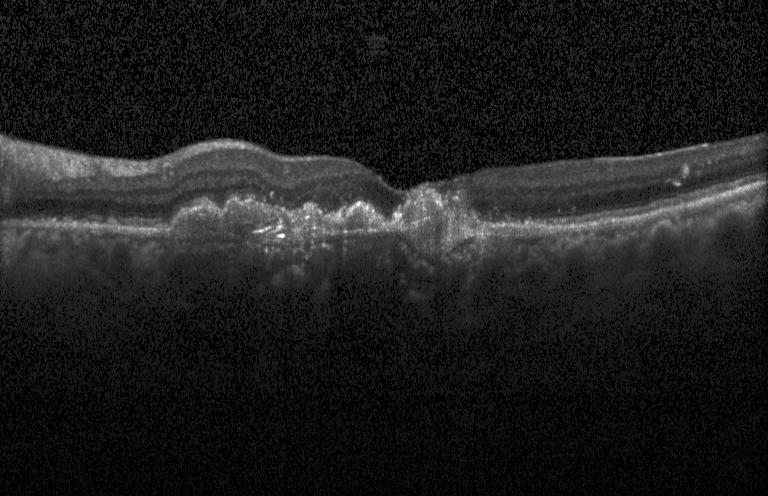

SD-OCT · retinal OCT B-scan · acquired on a Heidelberg Spectralis · centered on the fovea. Macular OCT: a choroidal neovascular membrane.